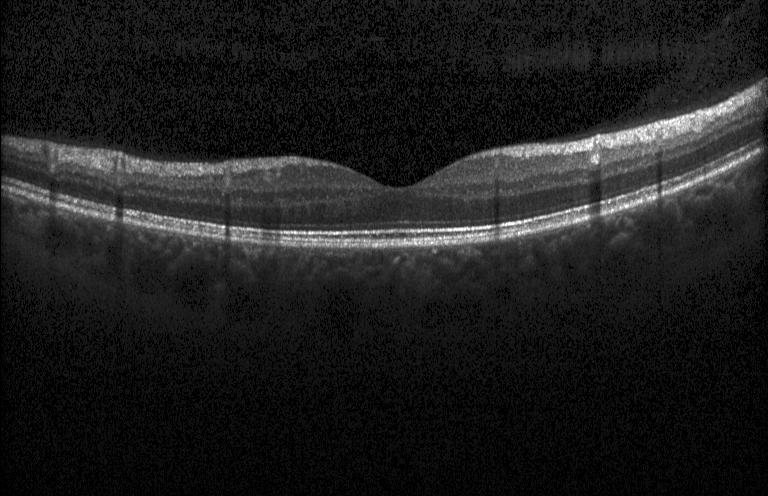 Optical coherence tomography scan; fovea-centered. Assessment: no choroidal neovascularization, diabetic macular edema, or drusen.